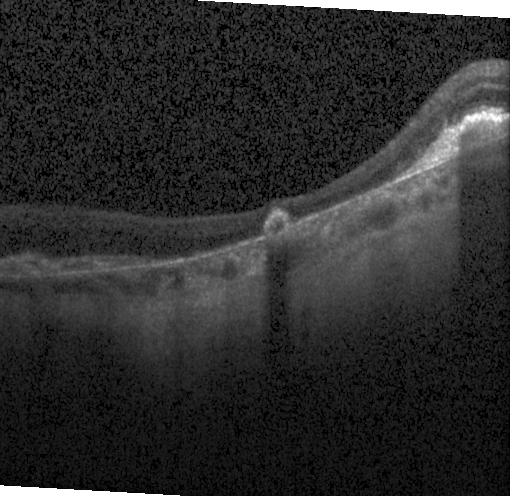 Heidelberg Spectralis OCT system · retinal OCT cross-section. Diagnosis: a choroidal neovascular membrane.